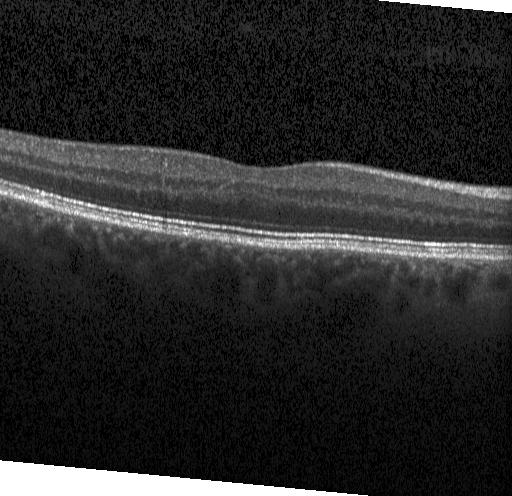 Spectral-domain optical coherence tomography. Optical coherence tomography B-scan. Through the macula. Instrument: Heidelberg Spectralis
The scan shows no choroidal neovascularization, diabetic macular edema, or drusen.